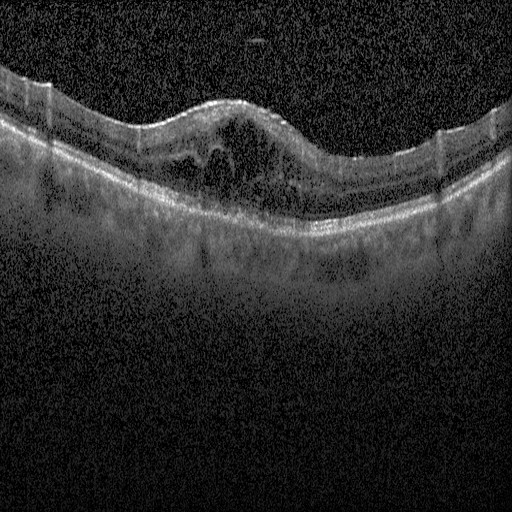 Instrument: Heidelberg Spectralis. Spectral-domain OCT. Optical coherence tomography B-scan. Horizontal scan through the fovea. Impression: diabetic macular edema.